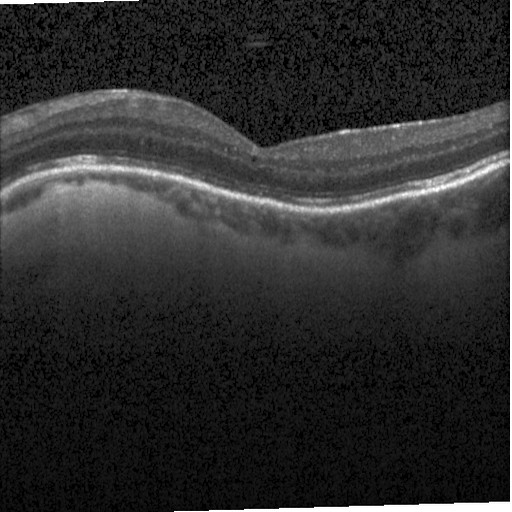

Macular OCT: diabetic macular edema (DME).